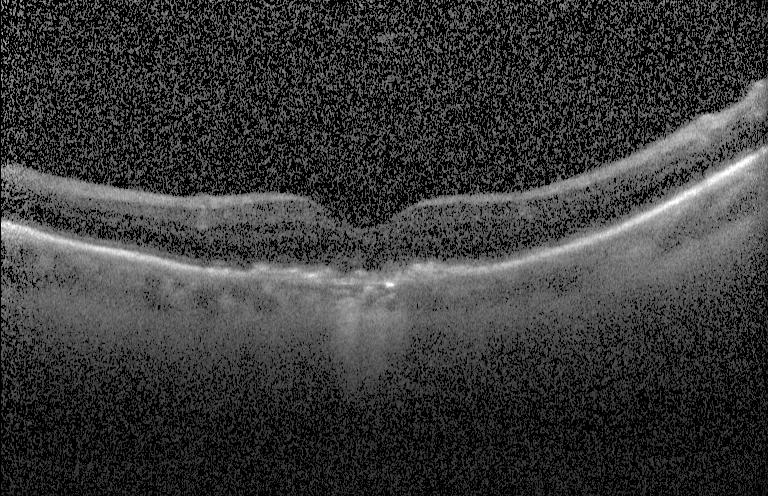

Diagnosis: choroidal neovascularization.